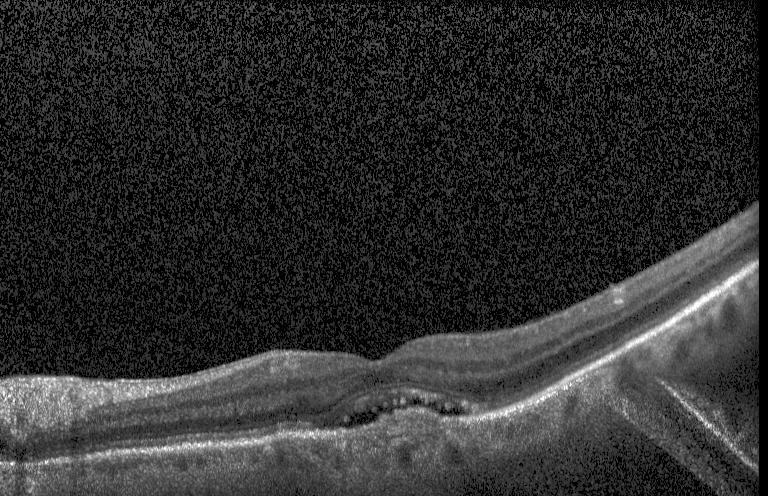
Macular scan; Heidelberg Spectralis; OCT line scan — This B-scan demonstrates a choroidal neovascular membrane.